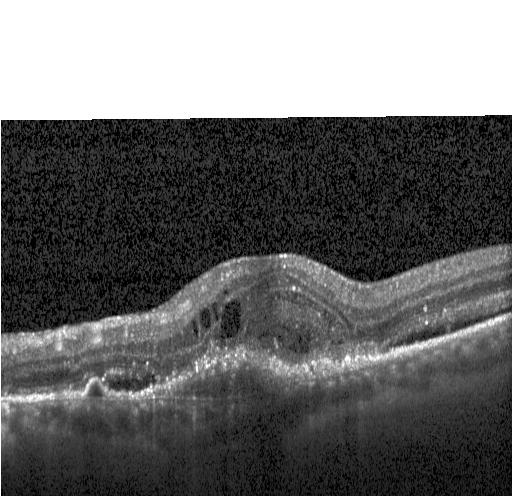

Spectral-domain OCT · retinal OCT B-scan.
Finding: CNV.